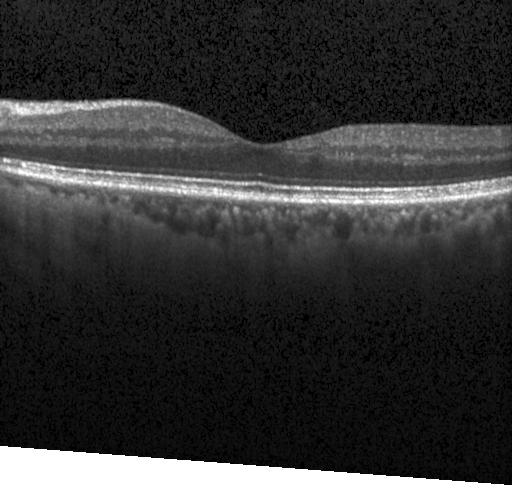

OCT B-scan showing no choroidal neovascularization, no diabetic macular edema, and no drusen.